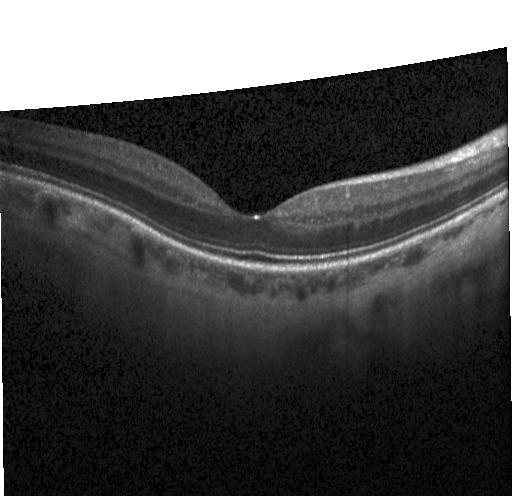

This B-scan demonstrates no CNV, no DME, and no drusen.